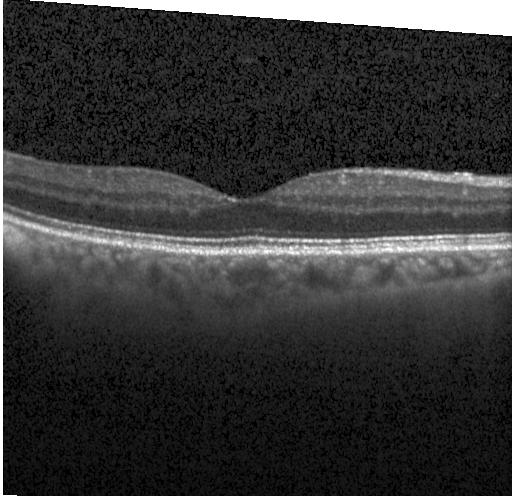

Optical coherence tomography scan. Heidelberg Spectralis OCT system. Macular scan. Spectral-domain optical coherence tomography. OCT finding: no choroidal neovascularization, diabetic macular edema, or drusen.